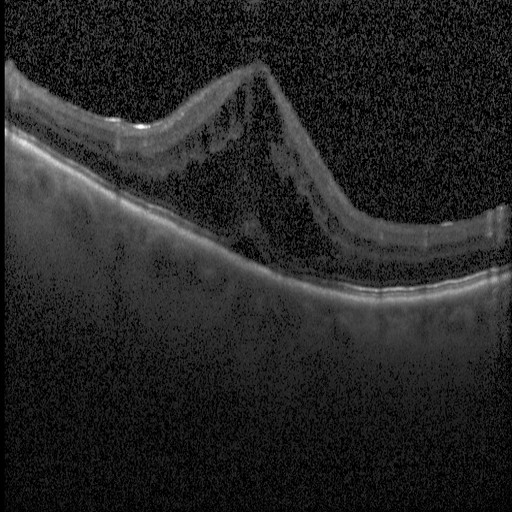 Through the macula · OCT line scan · spectral-domain optical coherence tomography · Heidelberg Spectralis OCT system — Assessment: DME.